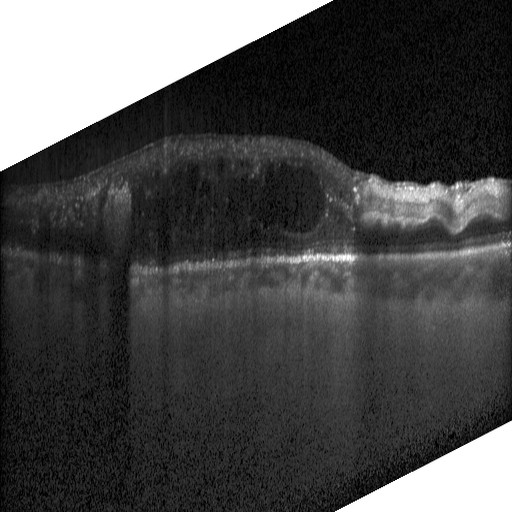

Spectral-domain OCT B-scan: diabetic macular edema (DME).